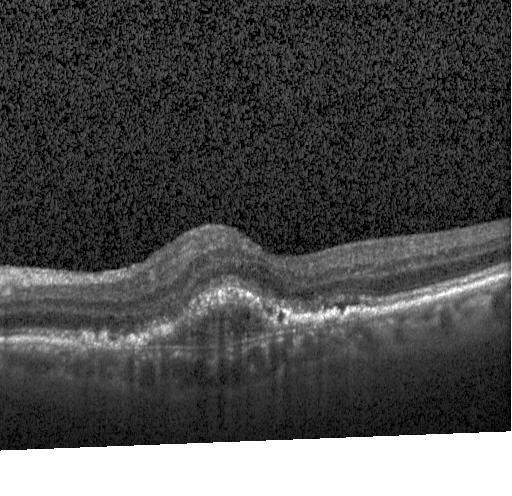
Macular OCT: choroidal neovascularization (CNV).